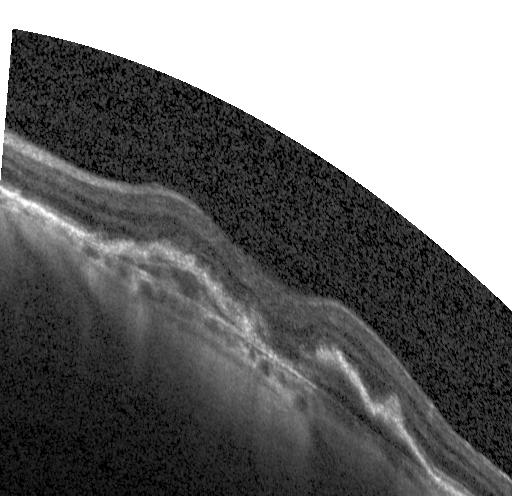

Retinal OCT B-scan · horizontal scan through the fovea · spectral-domain optical coherence tomography · Heidelberg Spectralis OCT system.
Dx: choroidal neovascularization (CNV).